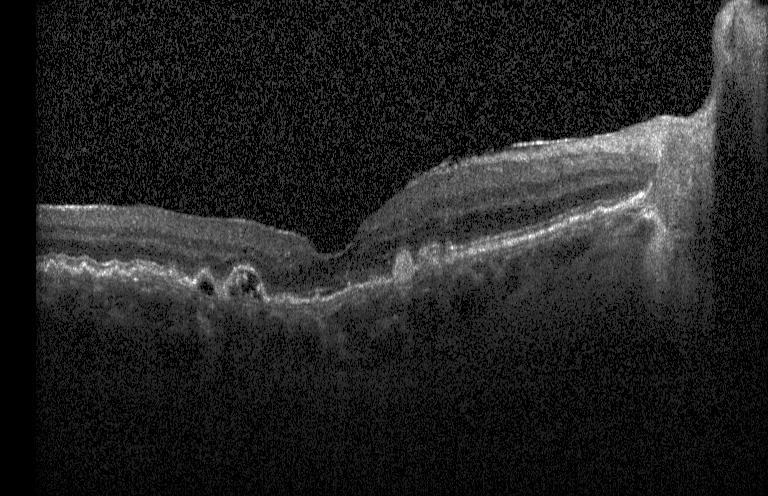
Retinal OCT B-scan — The scan shows a choroidal neovascular membrane.